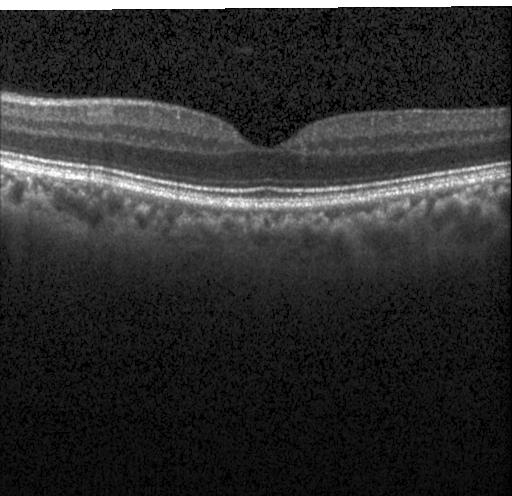

Retinal OCT cross-section. Horizontal scan through the fovea. Spectral-domain optical coherence tomography
This B-scan demonstrates no CNV, no DME, and no drusen.